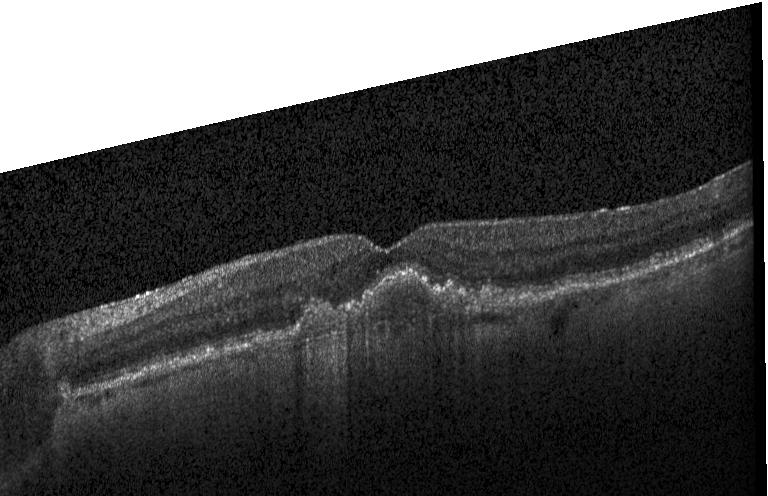

OCT line scan.
The scan shows choroidal neovascularization (CNV).